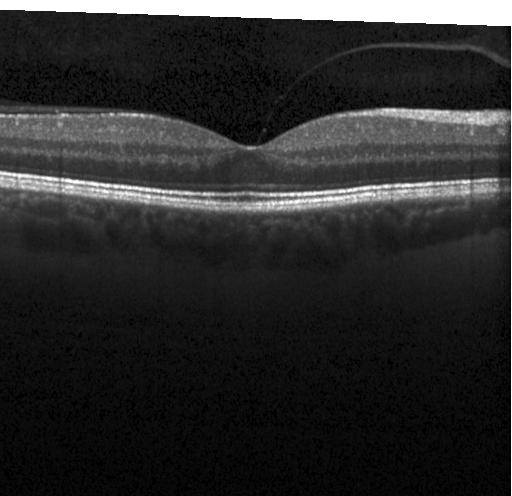

Centered on the fovea, SD-OCT, optical coherence tomography B-scan. Finding: no choroidal neovascularization, no diabetic macular edema, and no drusen.